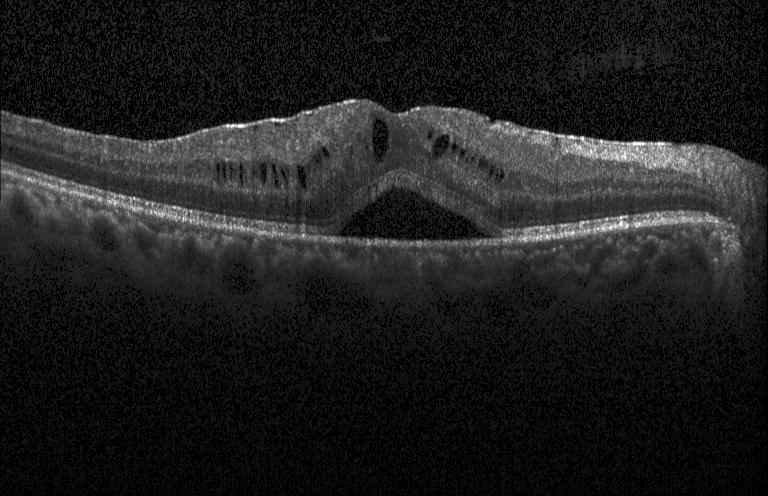
Through the macula · OCT B-scan · acquired on a Heidelberg Spectralis.
Diagnosis: diabetic macular edema.